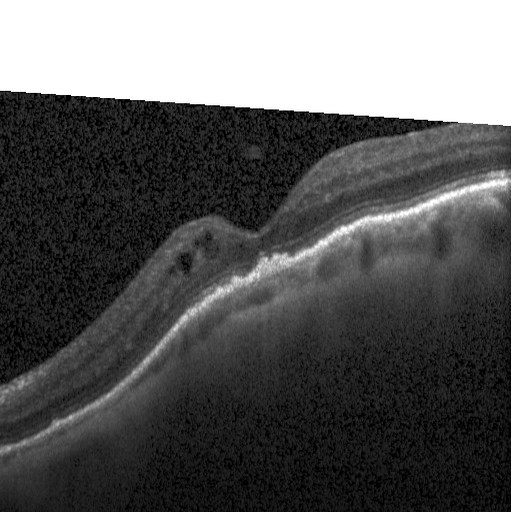
Optical coherence tomography scan. Centered on the fovea
Finding: diabetic macular edema (DME).